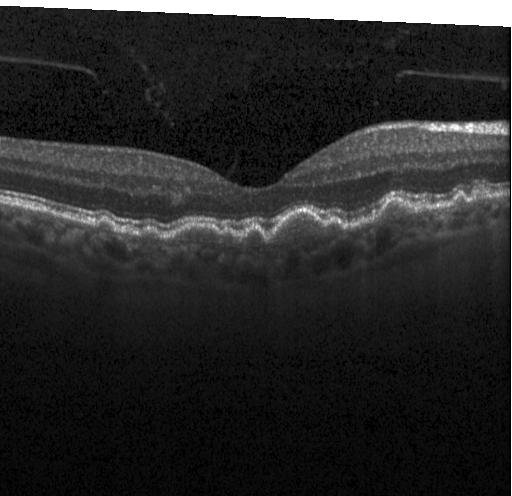
Spectral-domain optical coherence tomography. Acquired on a Heidelberg Spectralis. OCT B-scan — Macular OCT: sub-RPE drusenoid deposits.